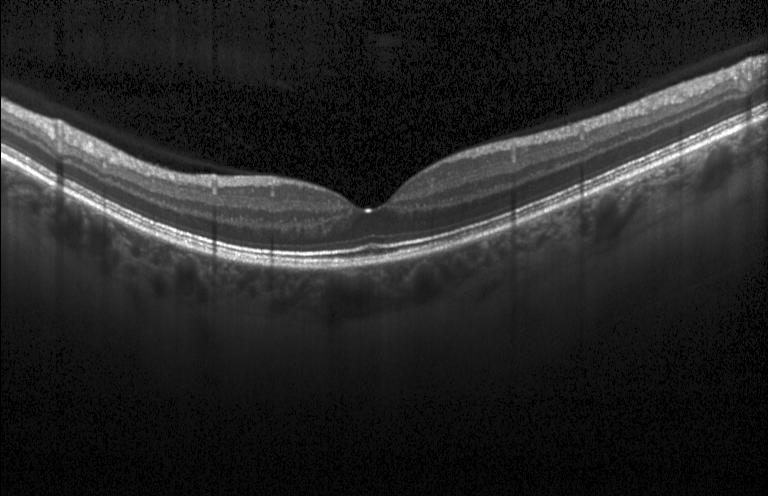
Centered on the fovea; retinal OCT B-scan.
The scan shows neither choroidal neovascularization, diabetic macular edema, nor drusen.